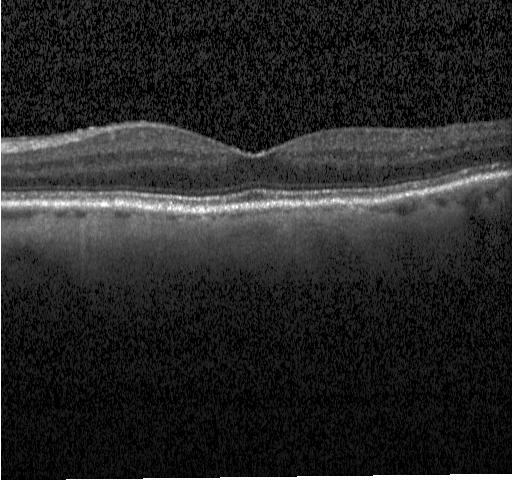

Diagnosis: no choroidal neovascularization, no diabetic macular edema, and no drusen.